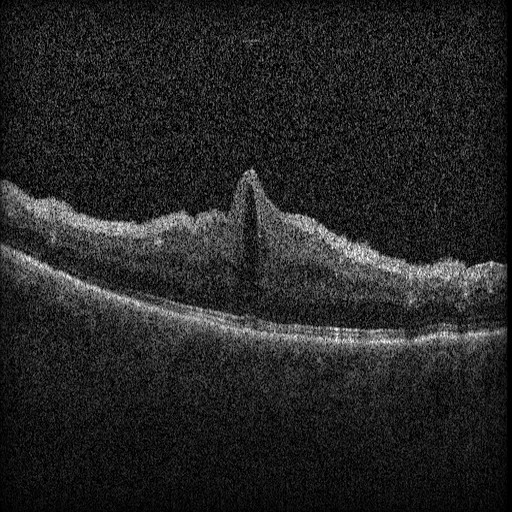
Optical coherence tomography scan · instrument: Heidelberg Spectralis · fovea-centered.
Finding: DME.